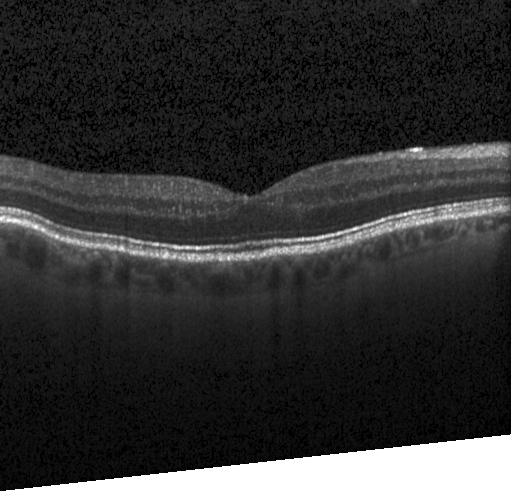 Impression: no CNV, DME, or drusen.